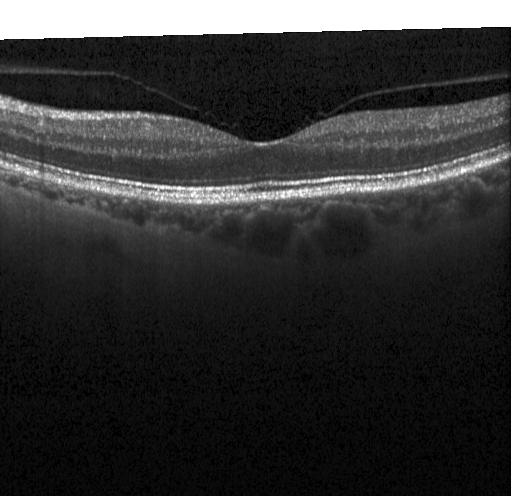

OCT B-scan showing no choroidal neovascularization, no diabetic macular edema, and no drusen.